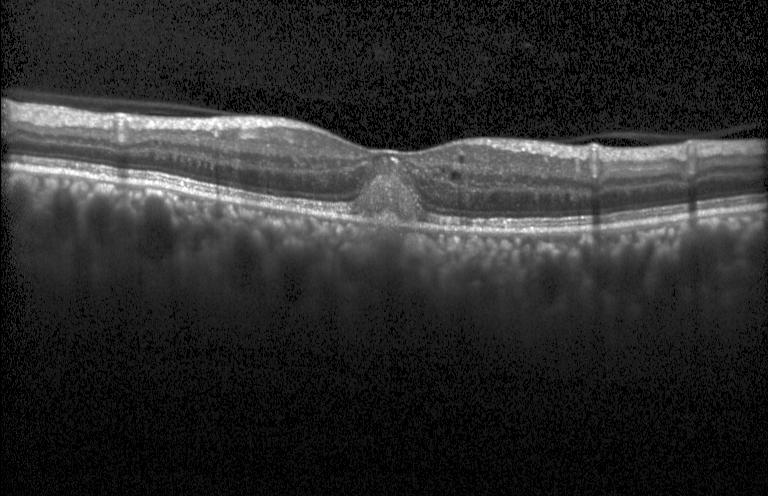
Spectral-domain OCT B-scan: a choroidal neovascular membrane.